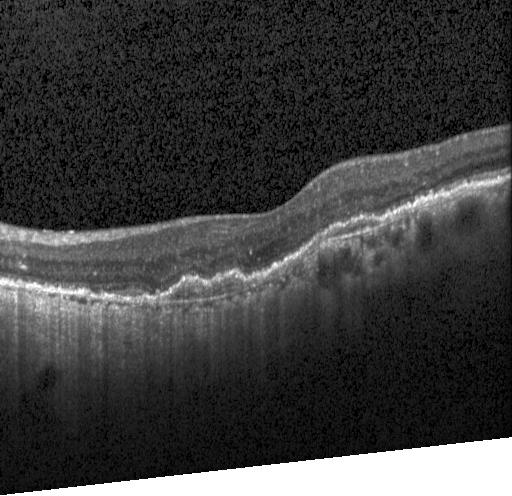
Retinal OCT B-scan · spectral-domain optical coherence tomography — A choroidal neovascular membrane.